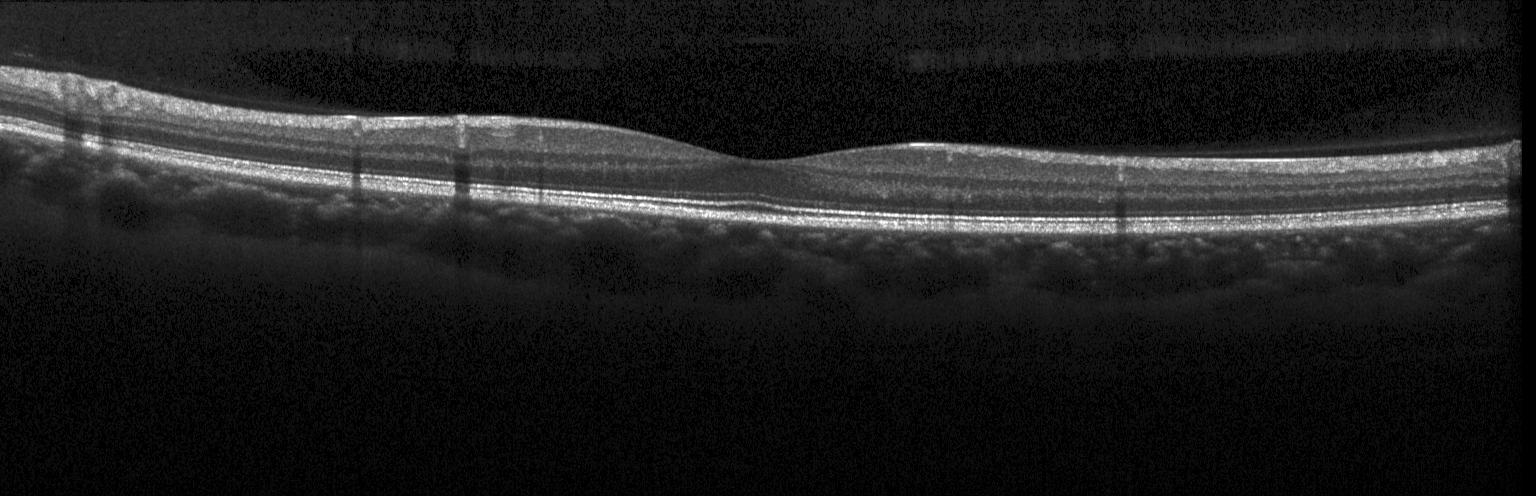

Heidelberg Spectralis. Optical coherence tomography B-scan. Impression: no choroidal neovascularization, no diabetic macular edema, and no drusen.